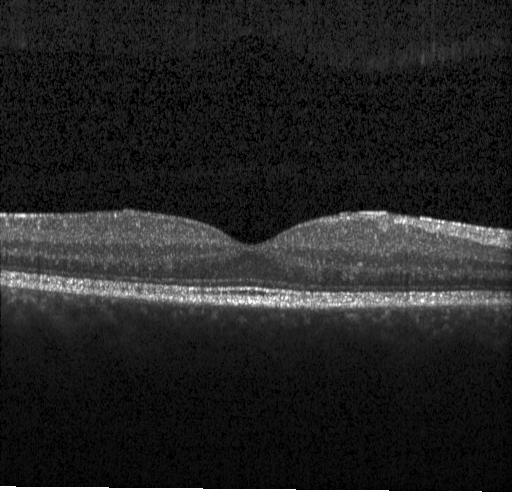 Retinal OCT cross-section — Finding: no choroidal neovascularization, diabetic macular edema, or drusen.